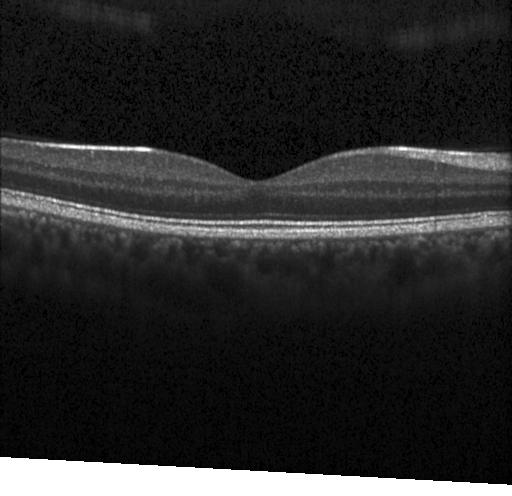

Diagnosis: neither choroidal neovascularization, diabetic macular edema, nor drusen.